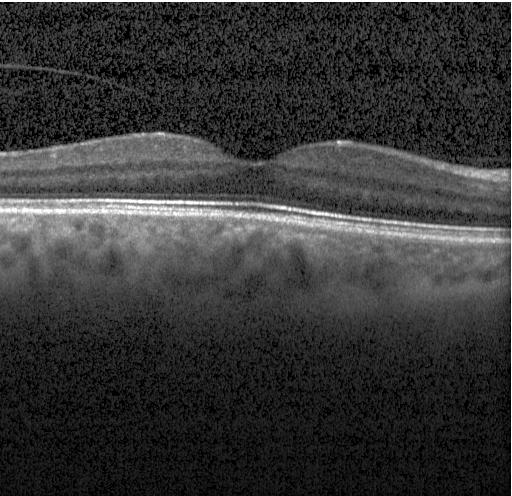 Optical coherence tomography B-scan. Diagnosis: no choroidal neovascularization, diabetic macular edema, or drusen.